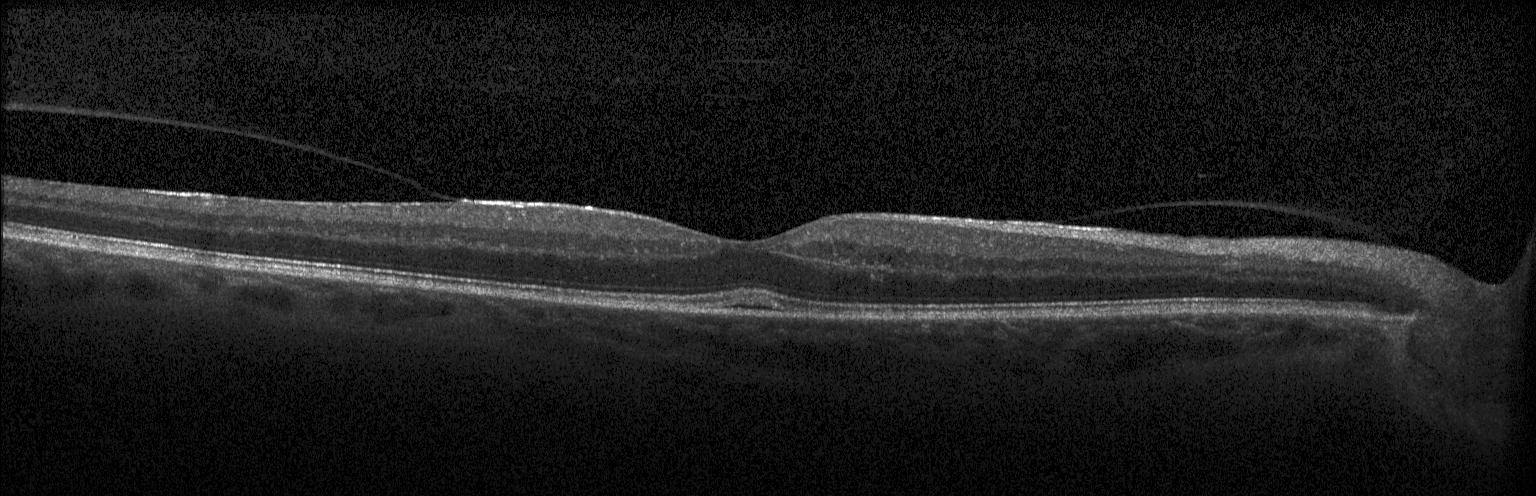

SD-OCT, retinal OCT B-scan. Assessment: no CNV, DME, or drusen.